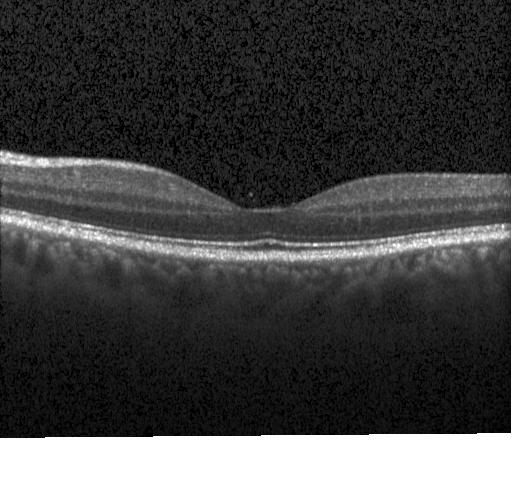 Through the macula · OCT line scan — This B-scan demonstrates no evidence of CNV, DME, or drusen.